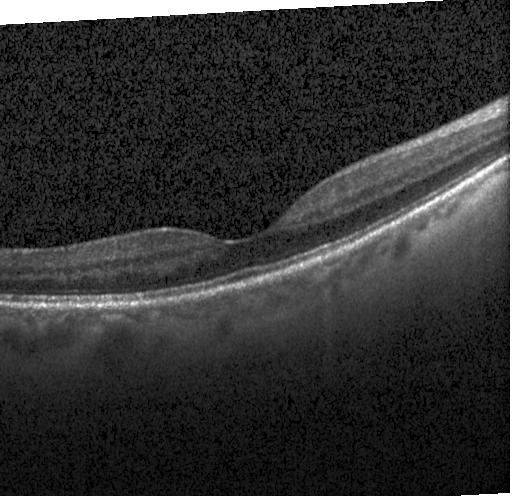
OCT finding: no choroidal neovascularization, diabetic macular edema, or drusen.